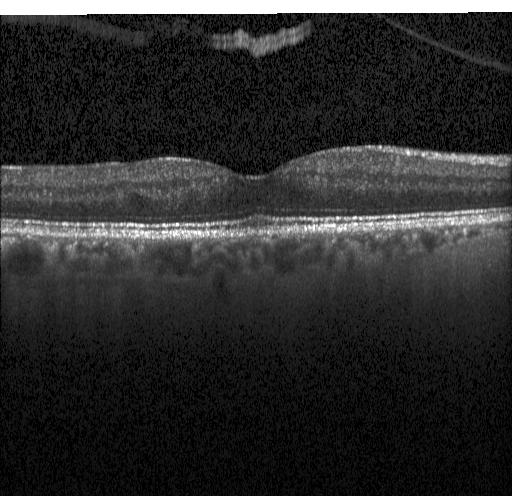

Spectral-domain OCT. Optical coherence tomography scan. Heidelberg Spectralis OCT system.
Diagnosis: no choroidal neovascularization, no diabetic macular edema, and no drusen.